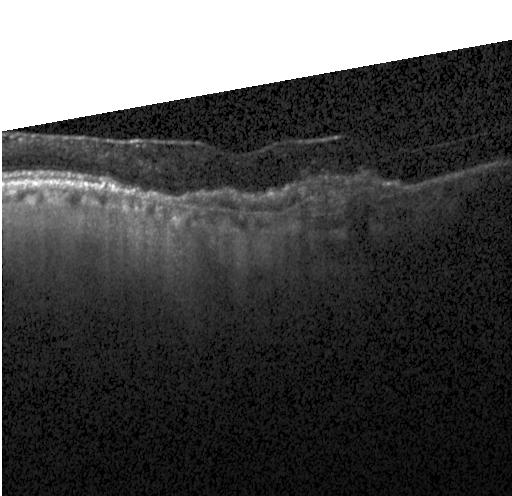 Centered on the fovea, Heidelberg Spectralis OCT system, retinal OCT B-scan, SD-OCT — Dx: choroidal neovascularization.